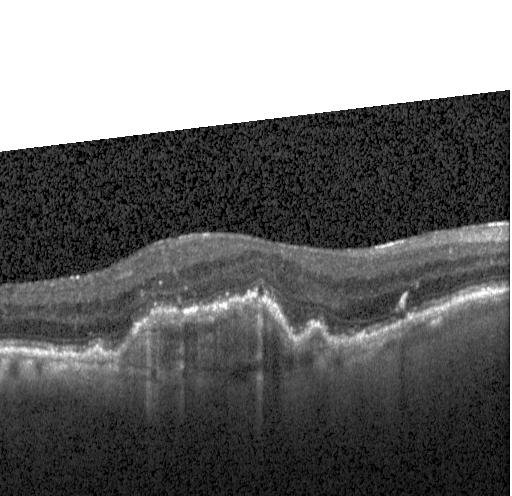
Instrument: Heidelberg Spectralis · optical coherence tomography B-scan · spectral-domain optical coherence tomography
The scan shows a choroidal neovascular membrane.